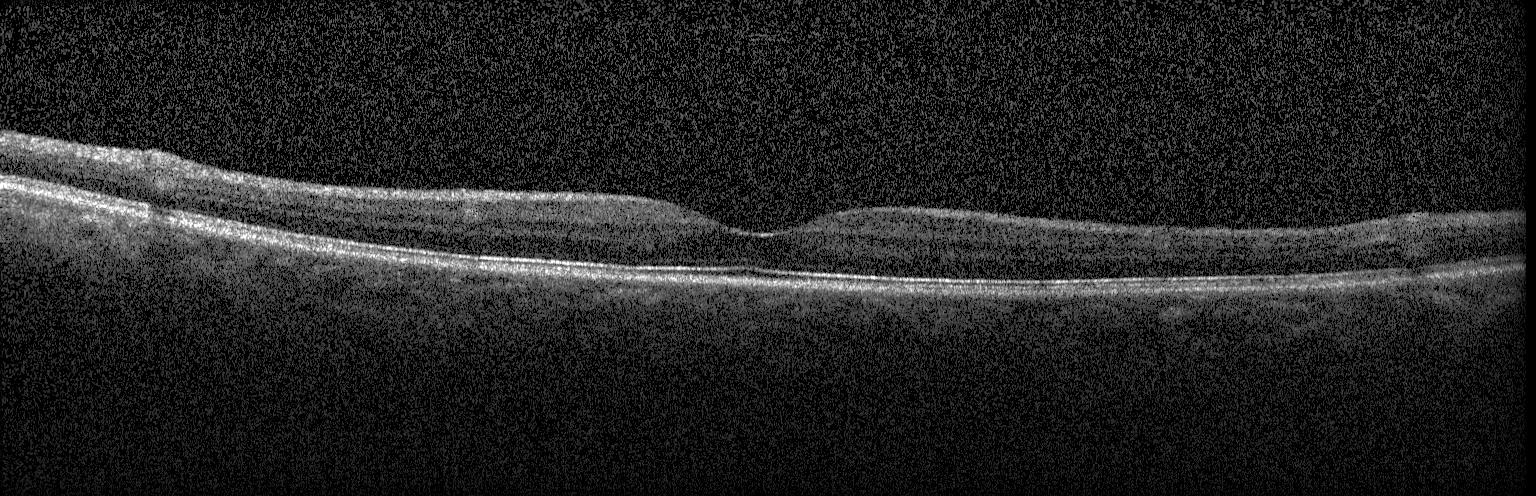
Retinal OCT cross-section showing no evidence of choroidal neovascularization, diabetic macular edema, or drusen.